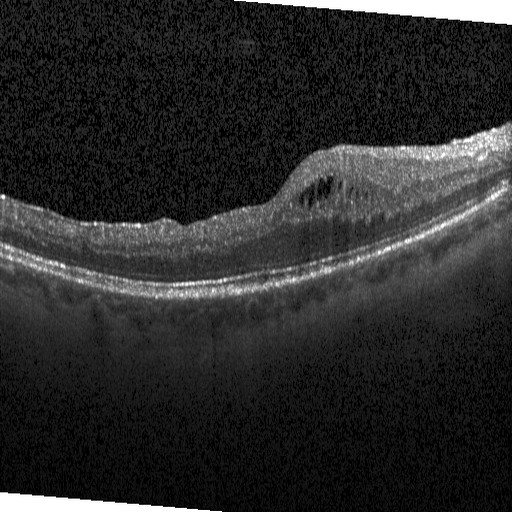

Heidelberg Spectralis; spectral-domain optical coherence tomography; retinal OCT B-scan; macular scan.
Assessment: diabetic macular edema.